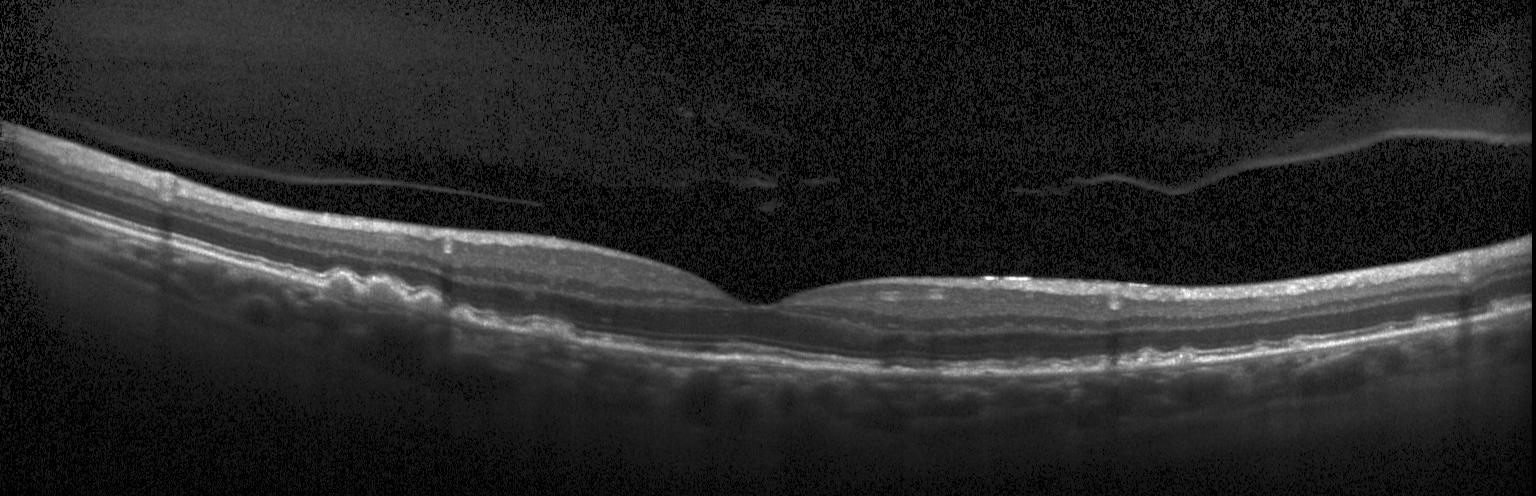 Optical coherence tomography B-scan — Dx: multiple drusen.